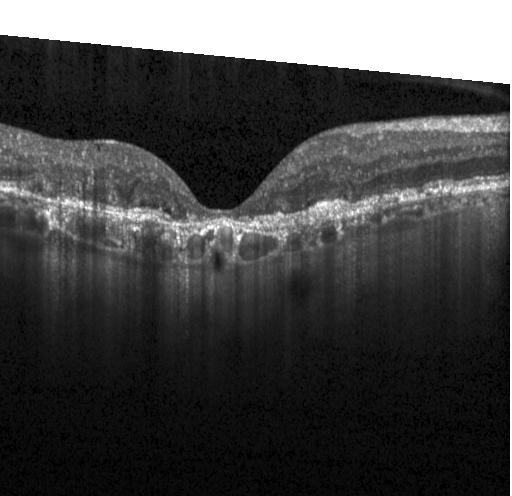 OCT B-scan showing a choroidal neovascular membrane.